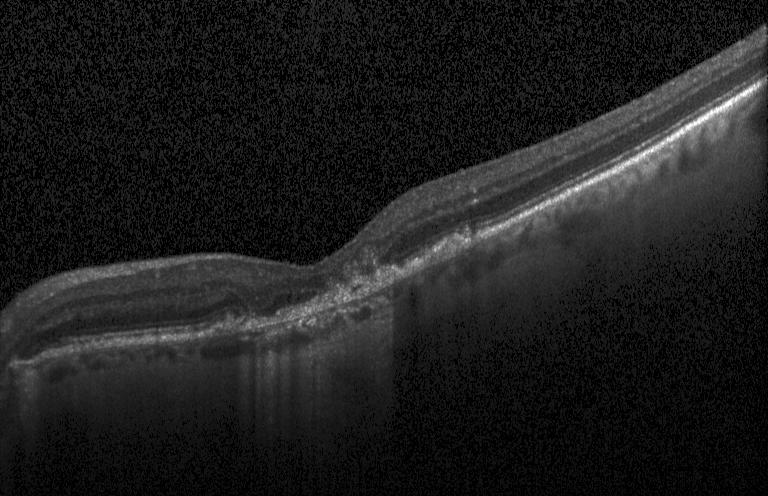
Optical coherence tomography B-scan · through the macula
Dx: CNV.